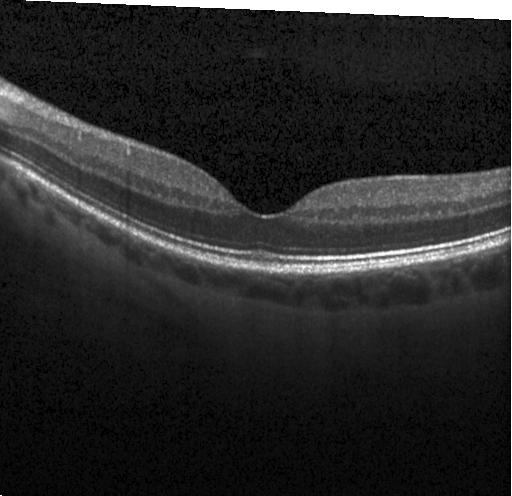

Retinal OCT cross-section, spectral-domain OCT
This B-scan demonstrates no choroidal neovascularization, no diabetic macular edema, and no drusen.